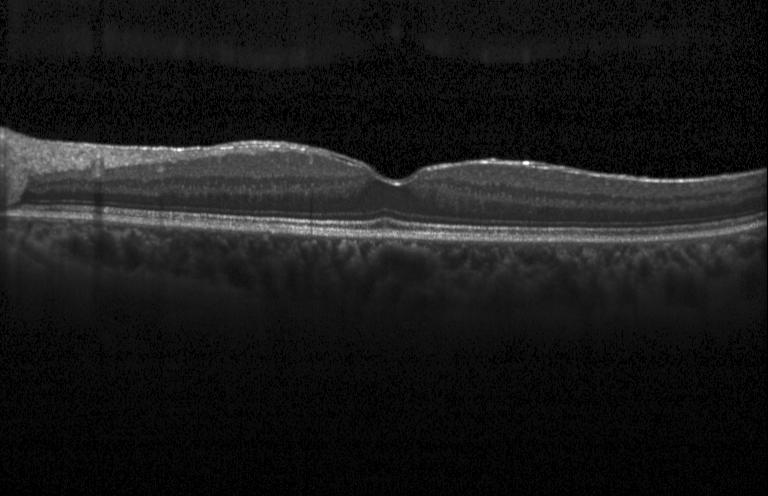

OCT line scan, Heidelberg Spectralis, centered on the fovea
Assessment: no choroidal neovascularization, no diabetic macular edema, and no drusen.